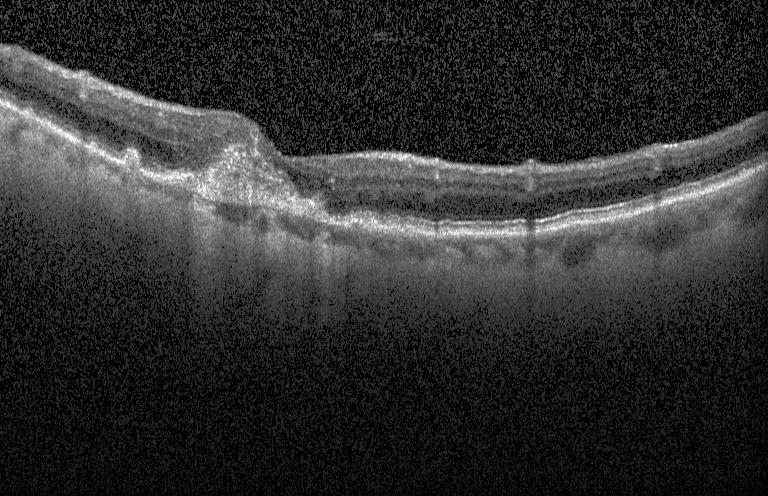
Finding: a choroidal neovascular membrane.